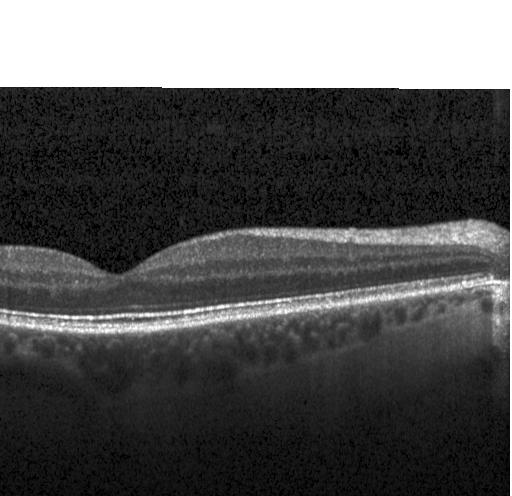

Spectral-domain optical coherence tomography. Through the macula. OCT line scan — This B-scan demonstrates no choroidal neovascularization, diabetic macular edema, or drusen.